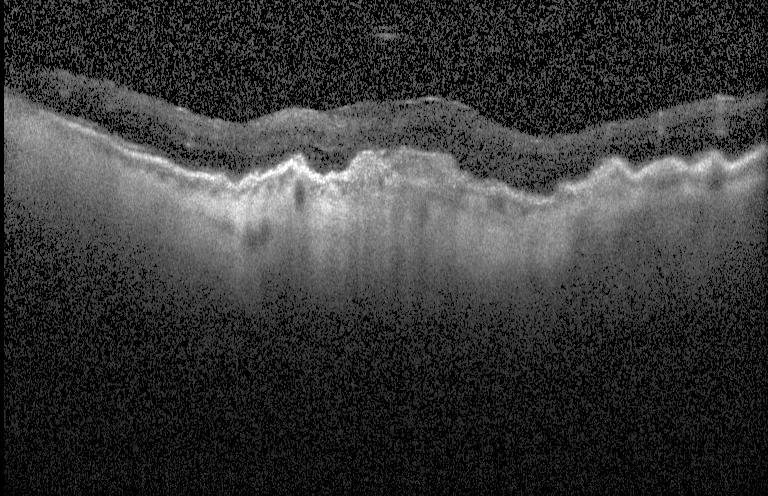 Diagnosis: a choroidal neovascular membrane.